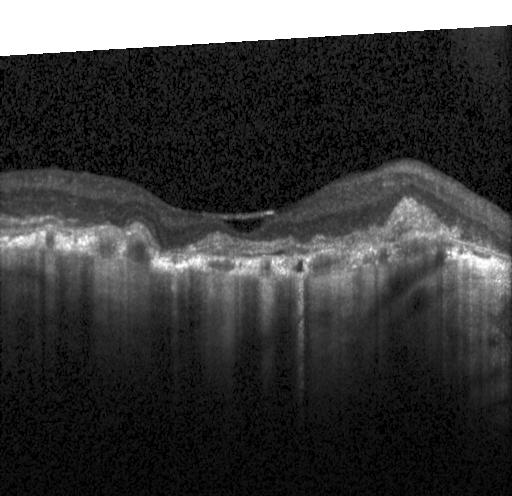

Spectral-domain optical coherence tomography. OCT B-scan.
Assessment: choroidal neovascularization (CNV).